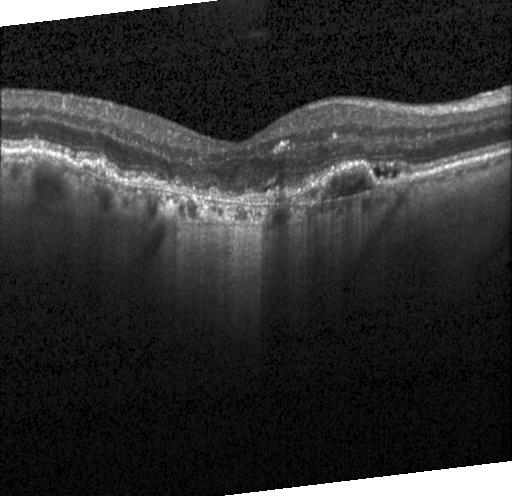
Retinal OCT cross-section showing a choroidal neovascular membrane.